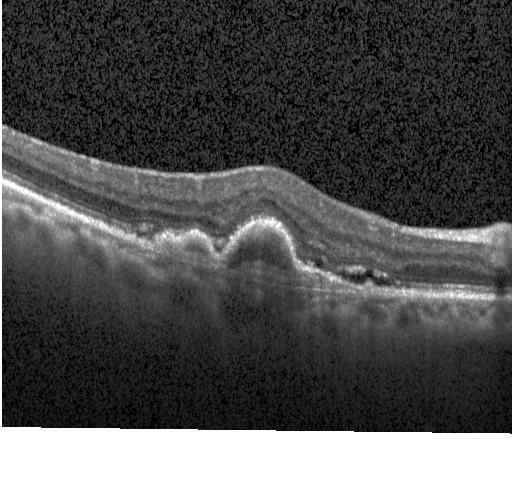

OCT line scan. Heidelberg Spectralis OCT system
The scan shows choroidal neovascularization (CNV).